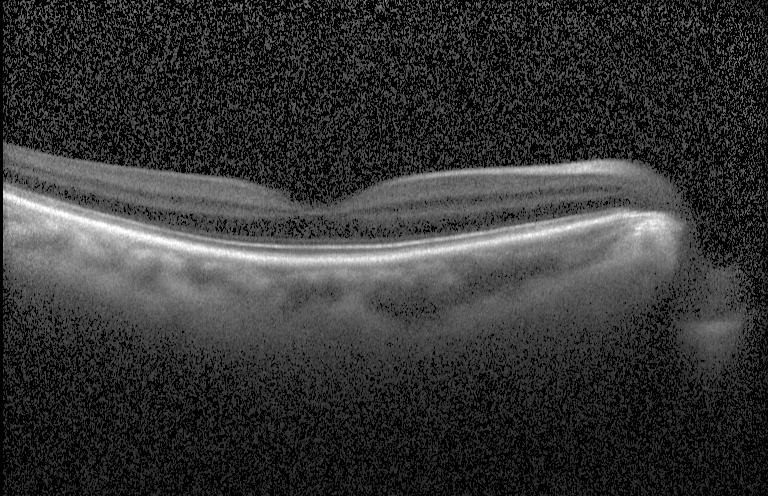
Acquired on a Heidelberg Spectralis · through the macula · optical coherence tomography B-scan · spectral-domain optical coherence tomography — Finding: no CNV, no DME, and no drusen.